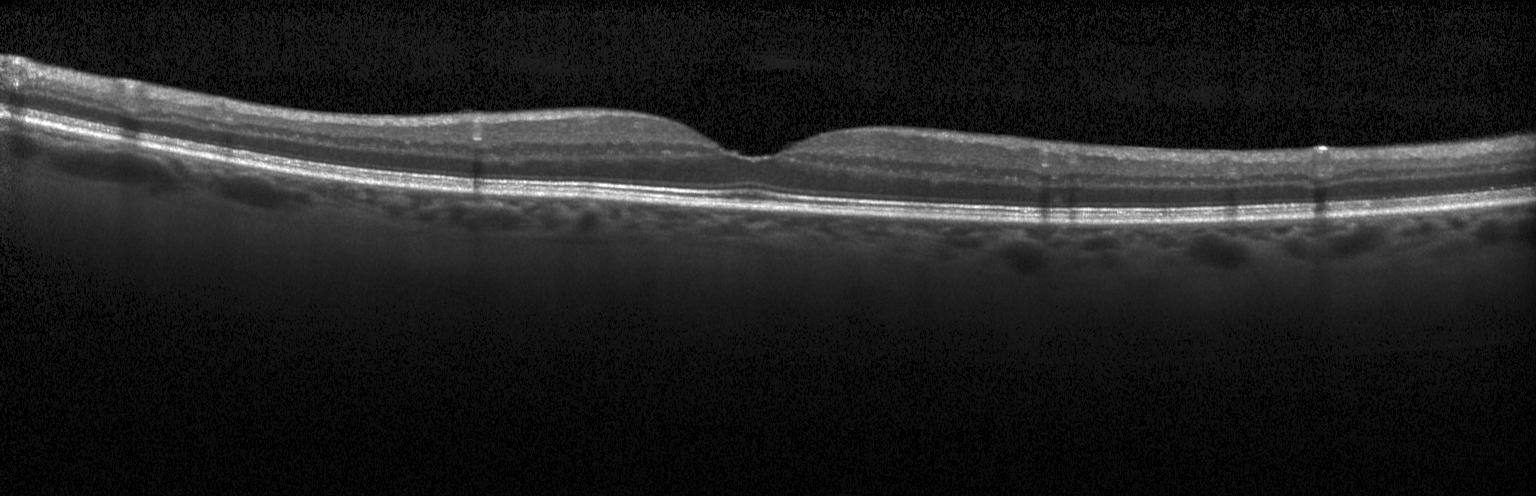
Impression: no evidence of choroidal neovascularization, diabetic macular edema, or drusen.